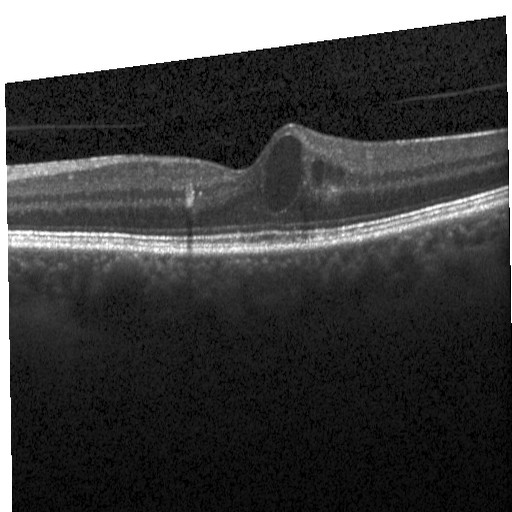
Spectral-domain OCT · OCT B-scan.
Diagnosis: diabetic macular edema (DME).